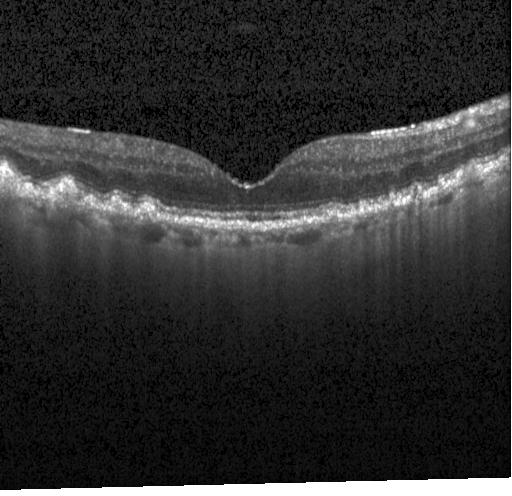

Retinal OCT B-scan, macular scan, acquired on a Heidelberg Spectralis.
OCT finding: multiple drusen.